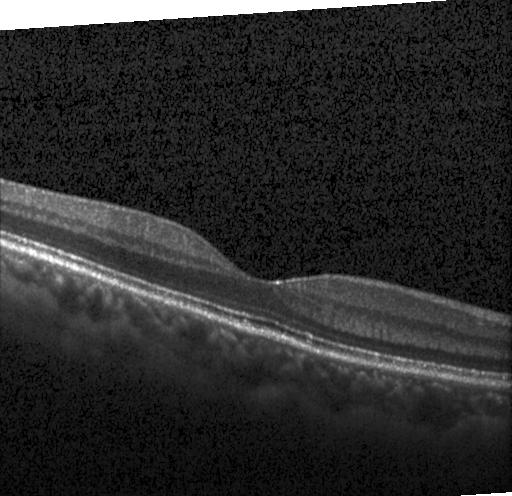
SD-OCT, optical coherence tomography scan, instrument: Heidelberg Spectralis, through the macula
Impression: no choroidal neovascularization, no diabetic macular edema, and no drusen.